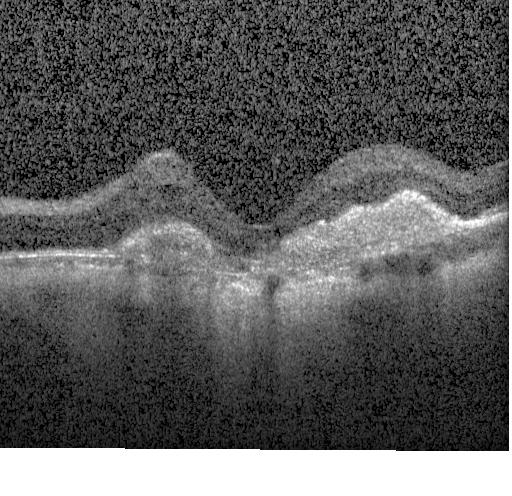

Centered on the fovea, Heidelberg Spectralis OCT system, spectral-domain optical coherence tomography, retinal OCT cross-section. Impression: choroidal neovascularization.